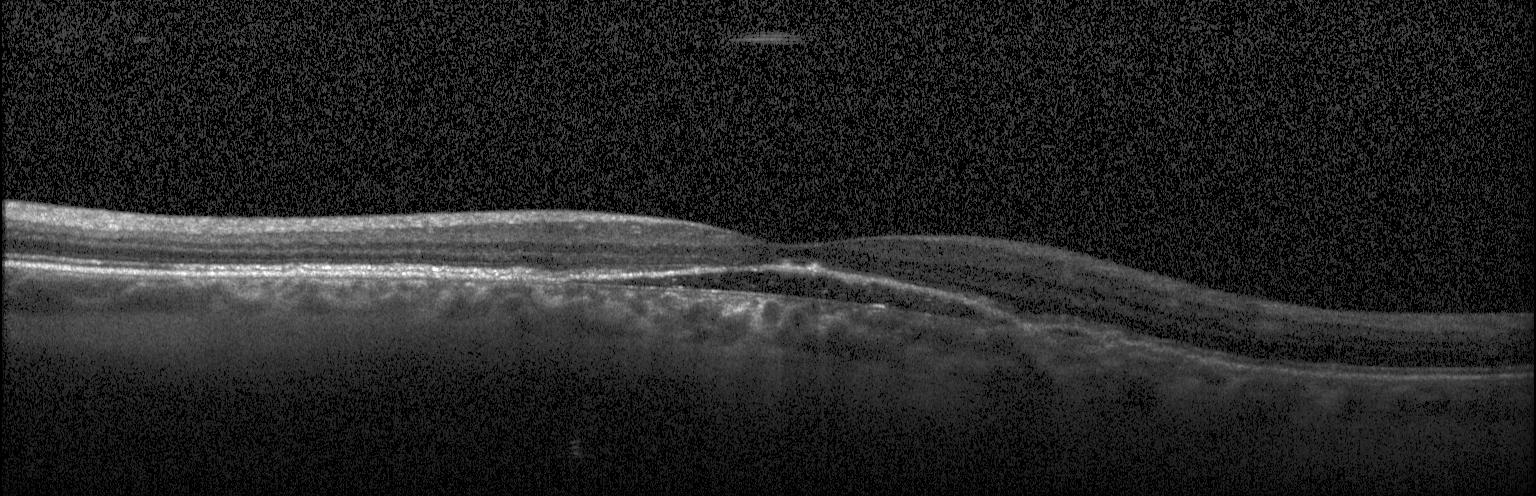

Heidelberg Spectralis OCT system · OCT line scan. Assessment: choroidal neovascularization.